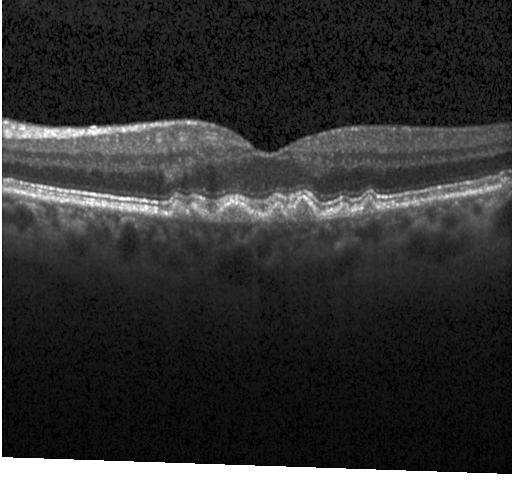 Sub-RPE drusenoid deposits.